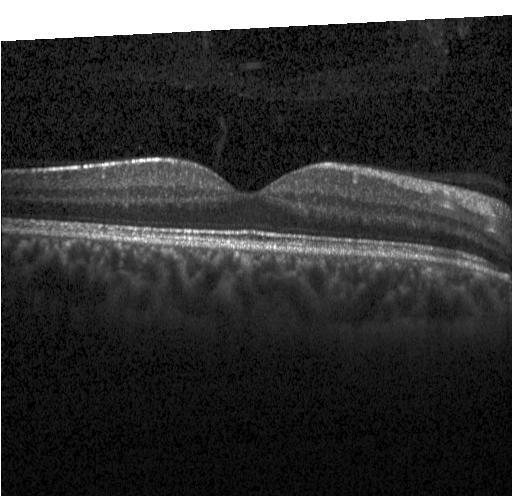 Spectral-domain OCT; centered on the fovea; OCT line scan; acquired on a Heidelberg Spectralis — Diagnosis: neither choroidal neovascularization, diabetic macular edema, nor drusen.